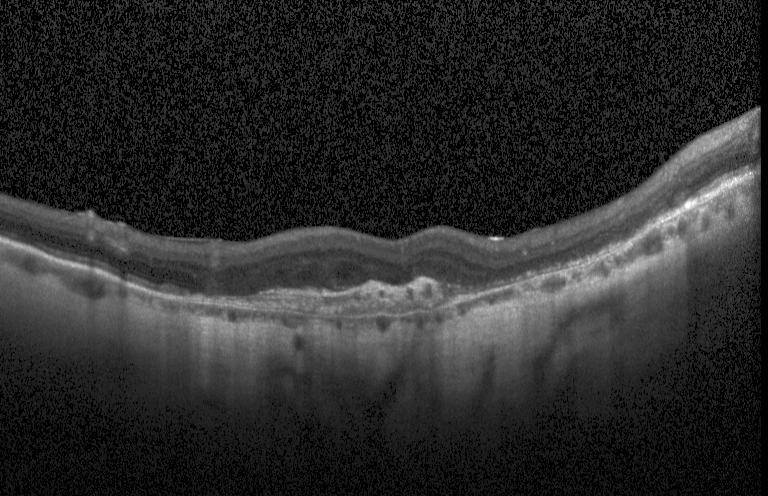
OCT B-scan. SD-OCT.
This B-scan demonstrates choroidal neovascularization.